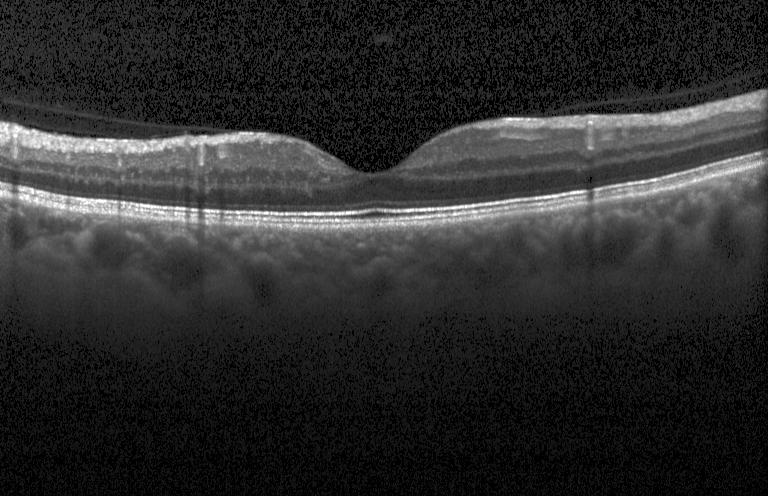
Spectral-domain OCT. OCT line scan.
Finding: neither choroidal neovascularization, diabetic macular edema, nor drusen.